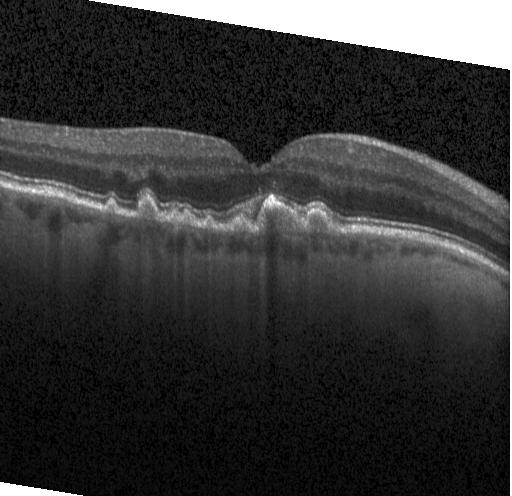
OCT B-scan. Impression: sub-RPE drusenoid deposits.